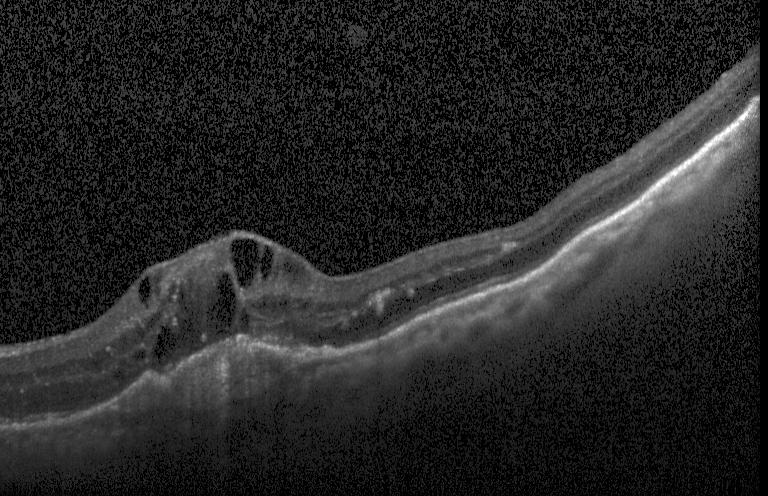

Retinal OCT cross-section; instrument: Heidelberg Spectralis; fovea-centered — Impression: choroidal neovascularization.